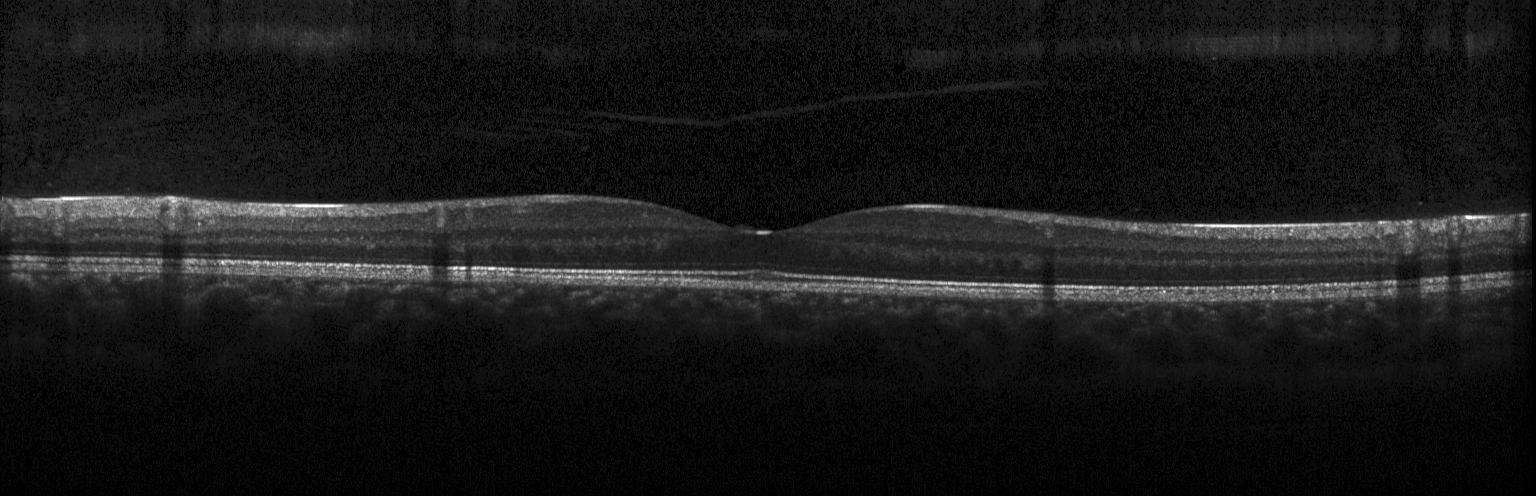 Diagnosis: no choroidal neovascularization, no diabetic macular edema, and no drusen.